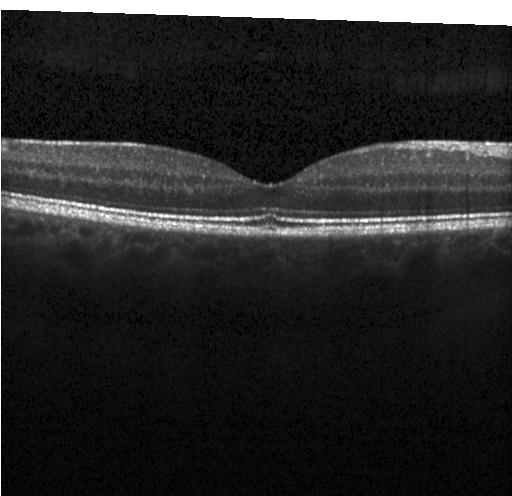

OCT line scan. OCT finding: no CNV, DME, or drusen.